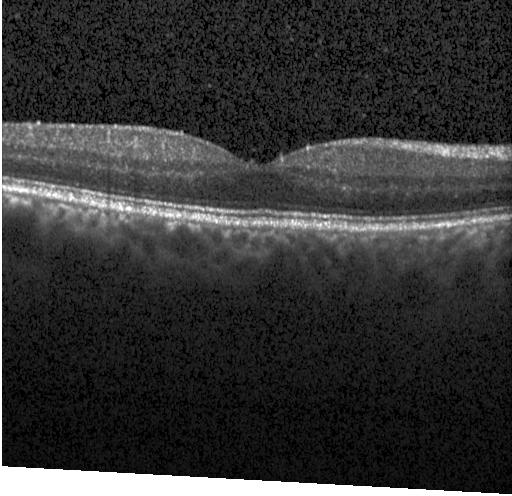 Impression: no evidence of CNV, DME, or drusen.